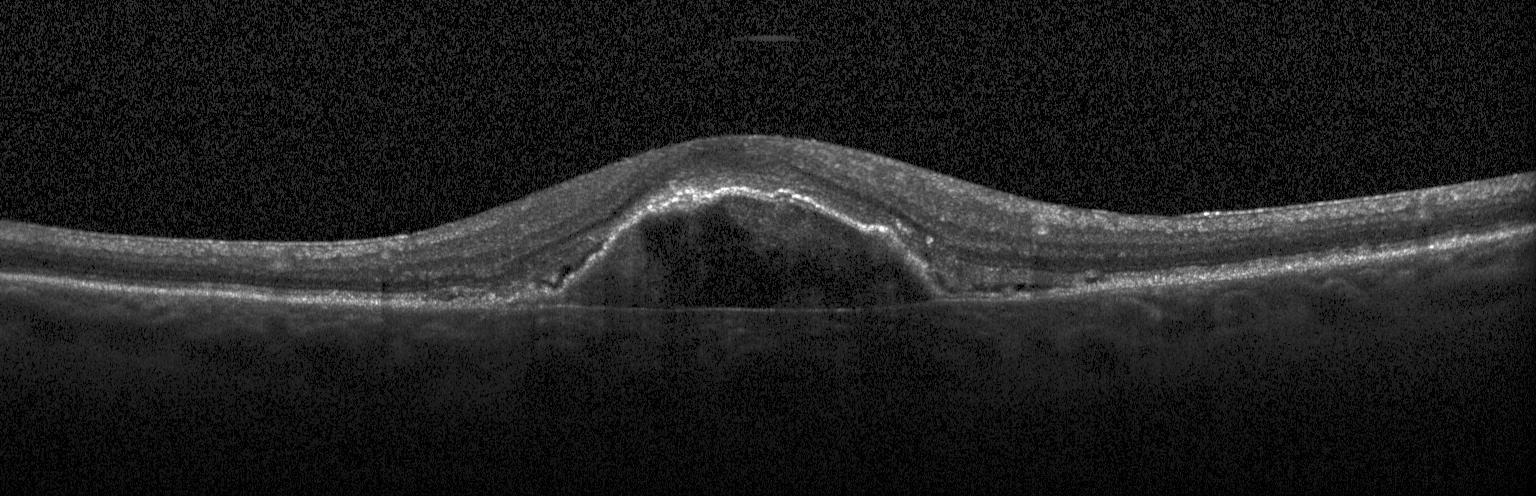 Macular OCT: a choroidal neovascular membrane.